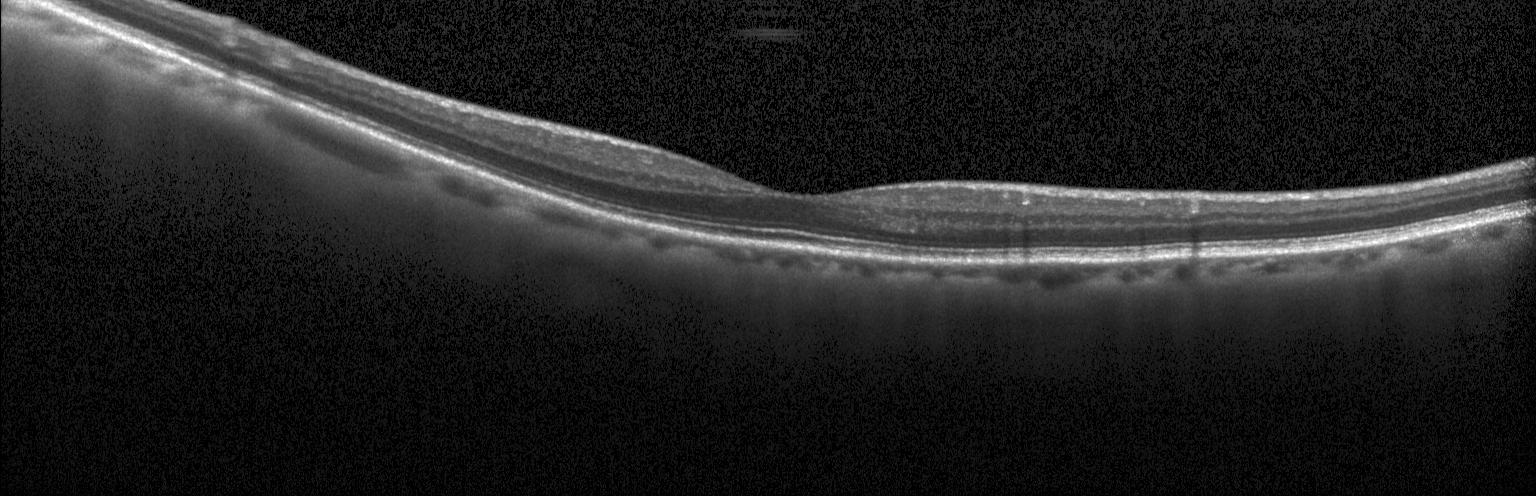

Spectral-domain OCT. OCT line scan
Diagnosis: no choroidal neovascularization, diabetic macular edema, or drusen.